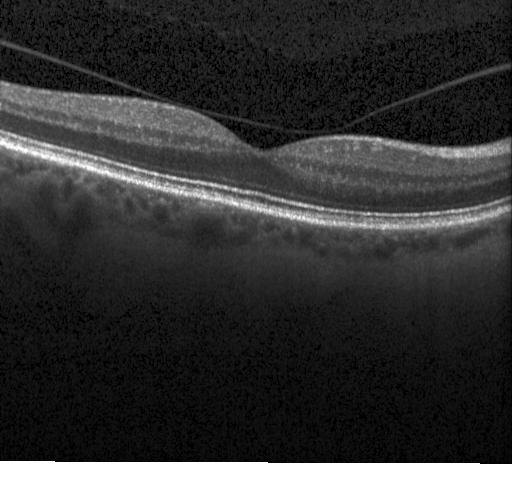 Spectral-domain OCT · acquired on a Heidelberg Spectralis · OCT line scan · macular scan. Macular OCT: no evidence of choroidal neovascularization, diabetic macular edema, or drusen.